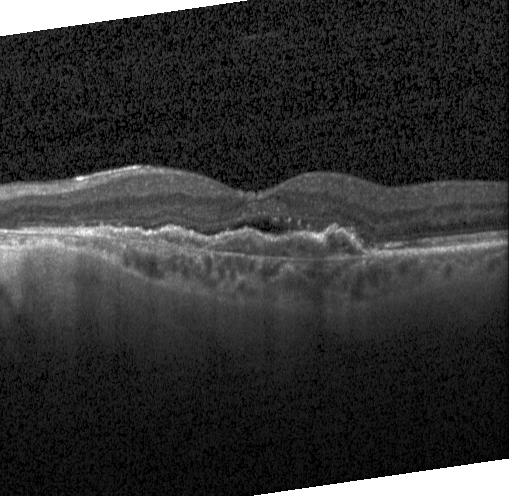
Retinal OCT B-scan. Horizontal scan through the fovea.
Diagnosis: a choroidal neovascular membrane.